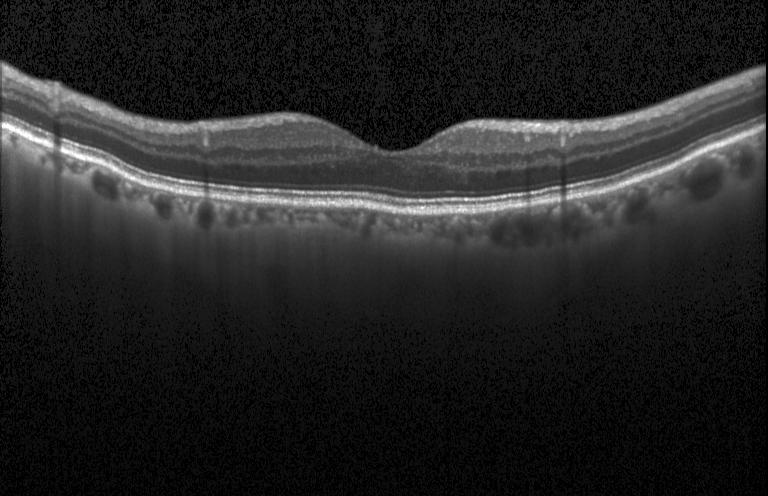
Neither choroidal neovascularization, diabetic macular edema, nor drusen.